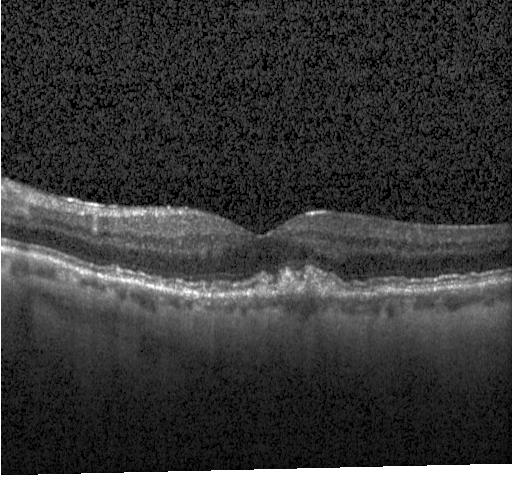

Optical coherence tomography scan. Centered on the fovea. Spectral-domain optical coherence tomography. Instrument: Heidelberg Spectralis — Drusen.